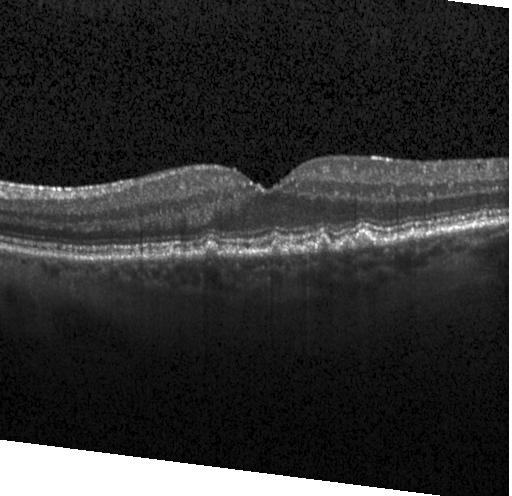 Retinal OCT B-scan, macular scan
Impression: multiple drusen.